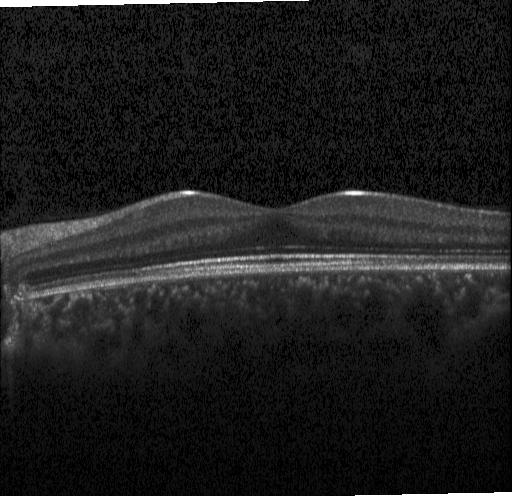 Retinal OCT B-scan — Diagnosis: neither CNV, DME, nor drusen.